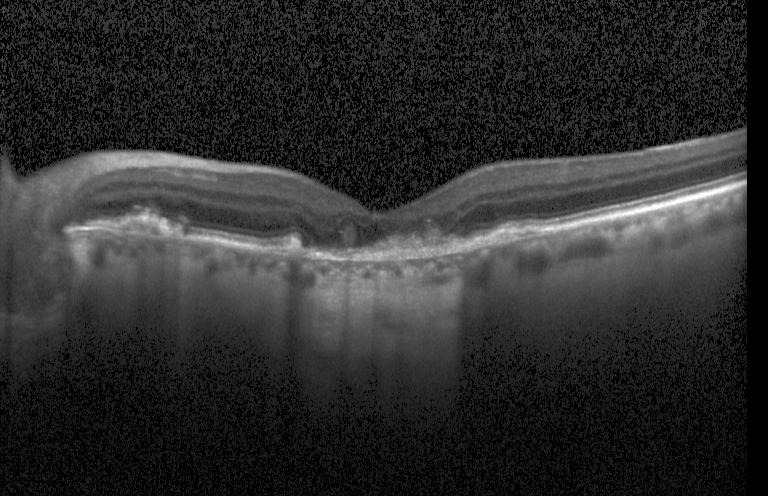

Spectral-domain OCT. Fovea-centered. Retinal OCT cross-section. Heidelberg Spectralis OCT system — This B-scan demonstrates a choroidal neovascular membrane.